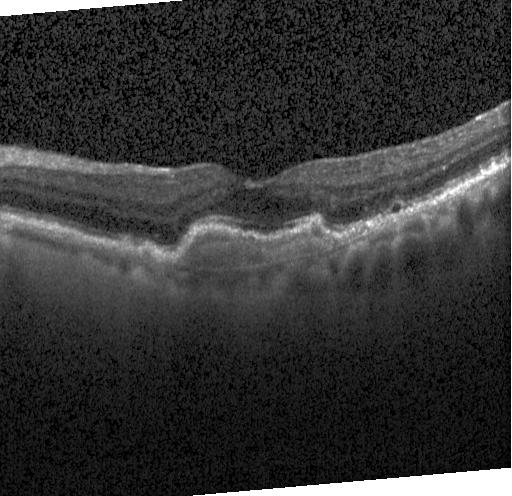
This B-scan demonstrates a choroidal neovascular membrane.